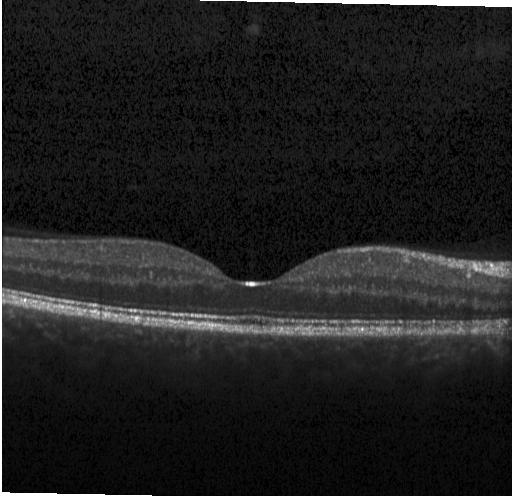

Retinal OCT B-scan
Dx: no evidence of choroidal neovascularization, diabetic macular edema, or drusen.